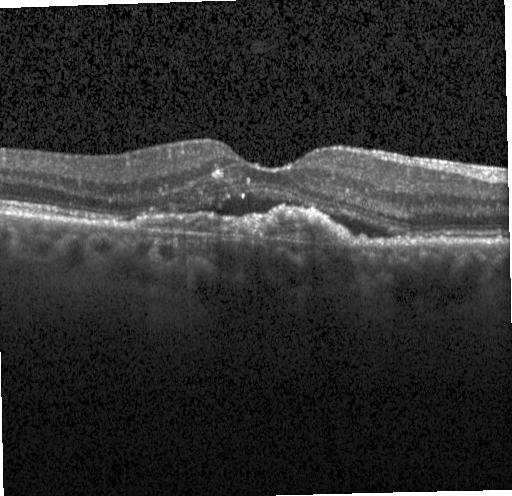

OCT B-scan showing a choroidal neovascular membrane.